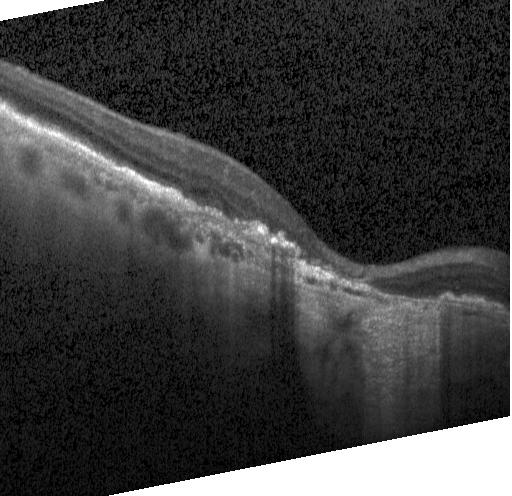 Retinal OCT B-scan; spectral-domain optical coherence tomography
This B-scan demonstrates choroidal neovascularization (CNV).